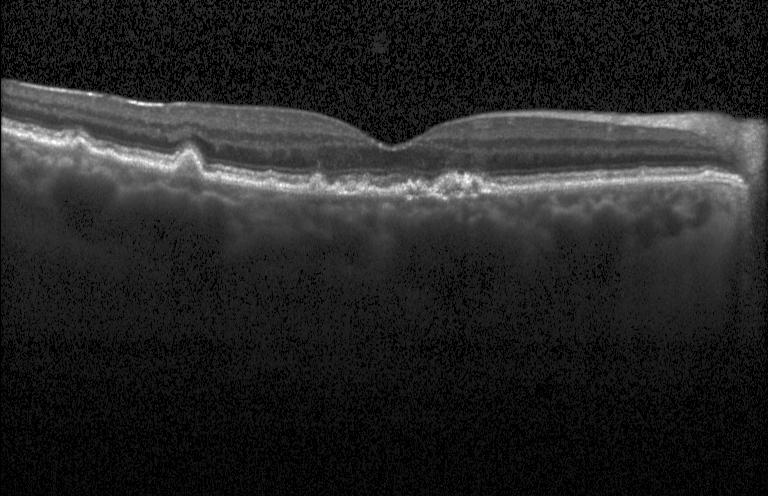

This B-scan demonstrates sub-RPE drusenoid deposits.